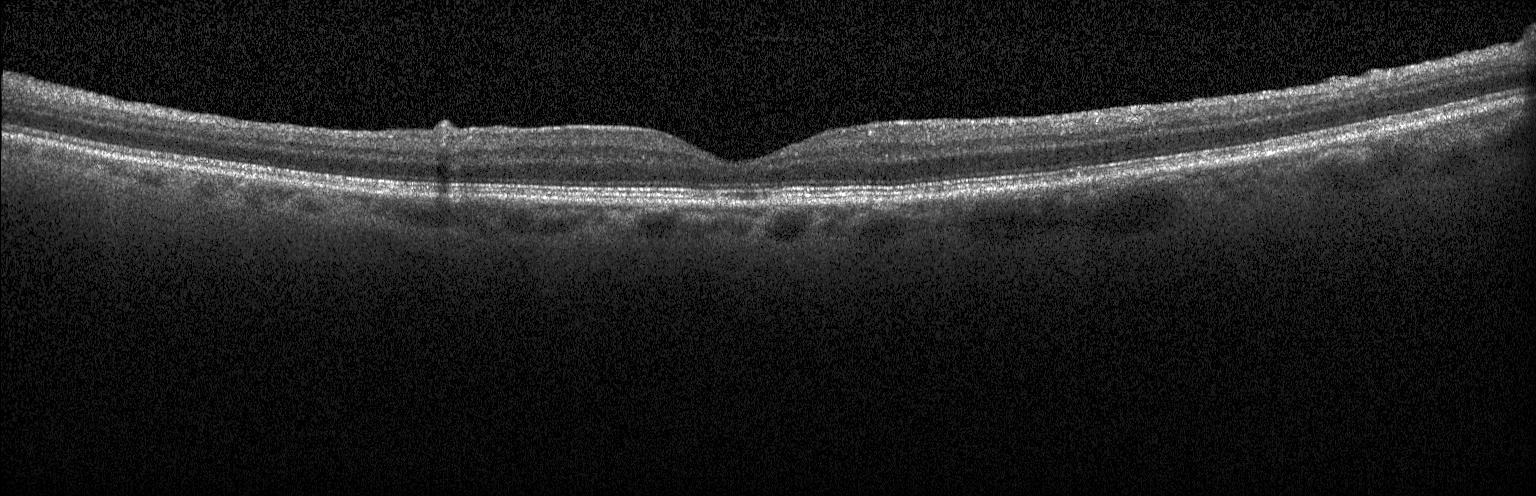 Finding: neither choroidal neovascularization, diabetic macular edema, nor drusen.